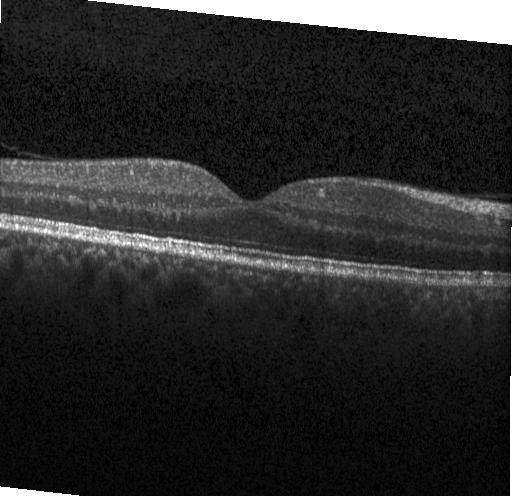
Acquired on a Heidelberg Spectralis, through the macula, OCT line scan.
Assessment: no choroidal neovascularization, no diabetic macular edema, and no drusen.